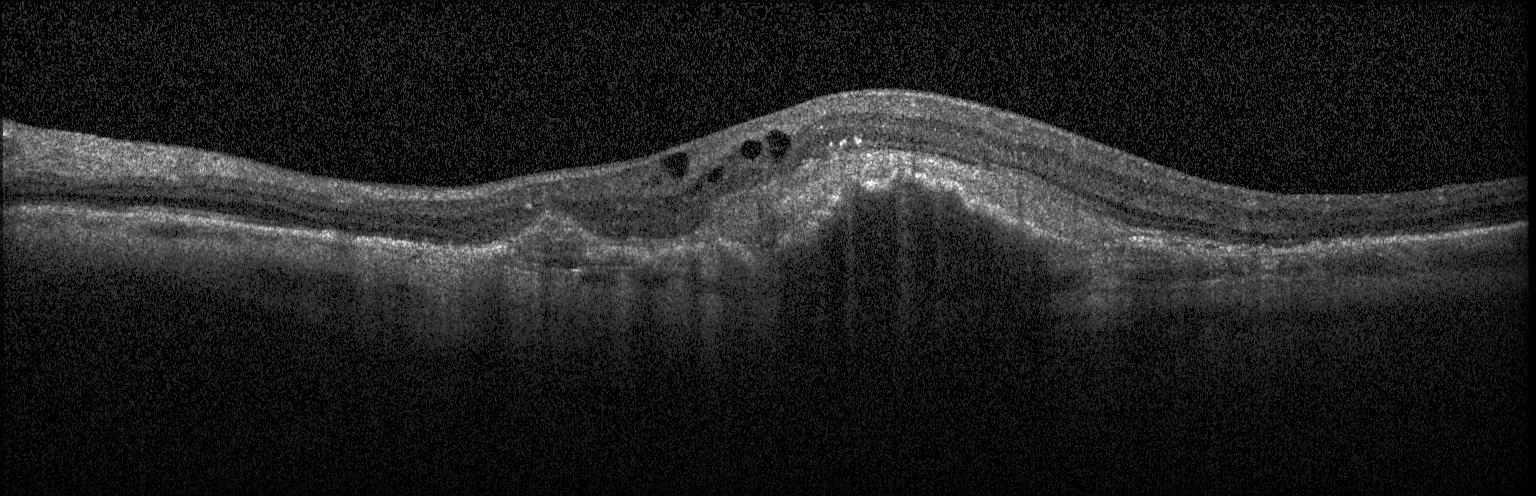 Horizontal scan through the fovea; Heidelberg Spectralis OCT system; spectral-domain OCT; optical coherence tomography B-scan — Diagnosis: choroidal neovascularization (CNV).